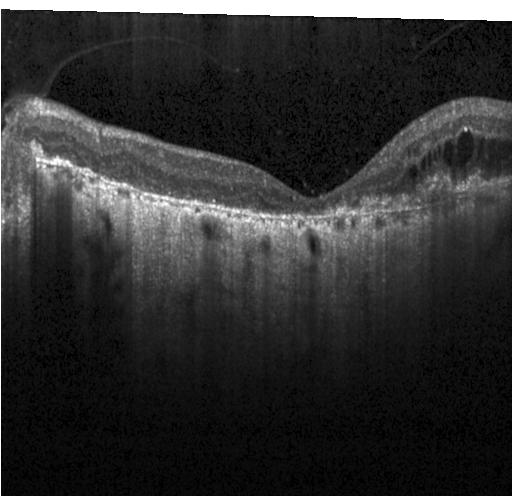
Retinal OCT cross-section — Macular OCT: CNV.